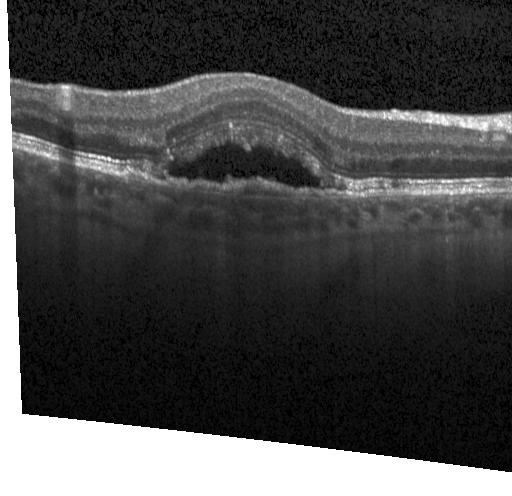
This B-scan demonstrates CNV.